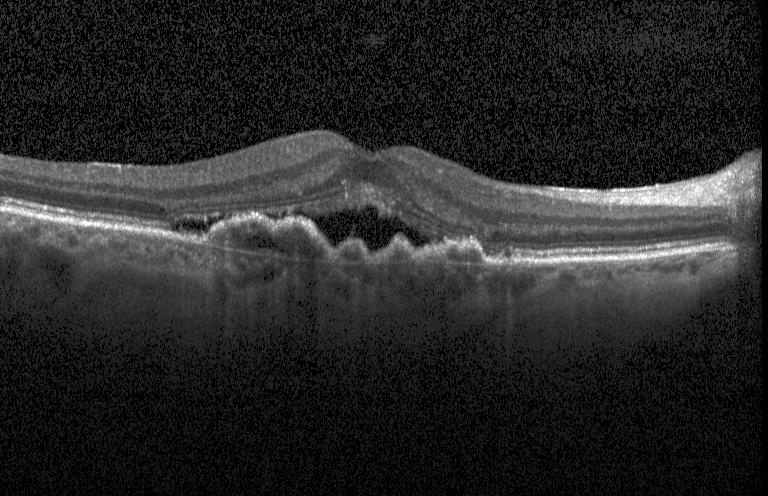 OCT line scan. Spectral-domain OCT. Dx: a choroidal neovascular membrane.